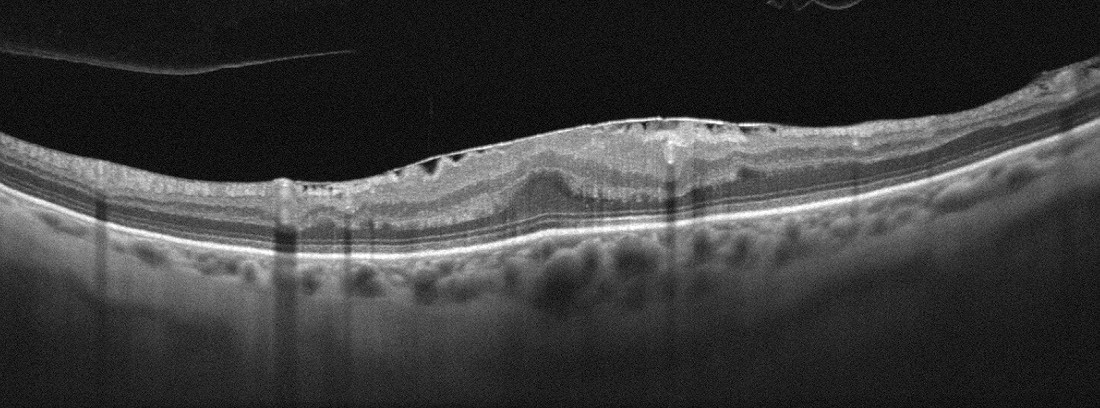
Finding: epiretinal membrane (ERM).